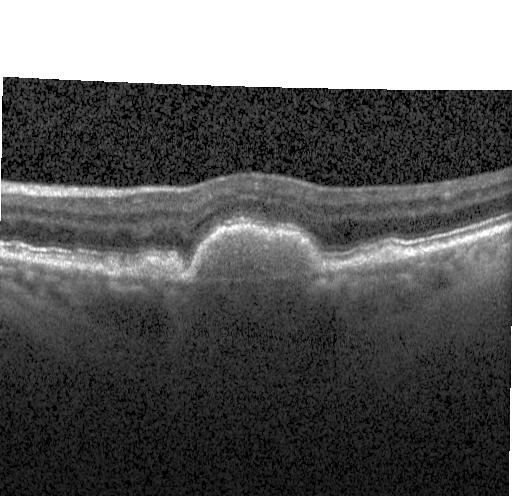

Optical coherence tomography scan. Spectral-domain optical coherence tomography. The scan shows CNV.